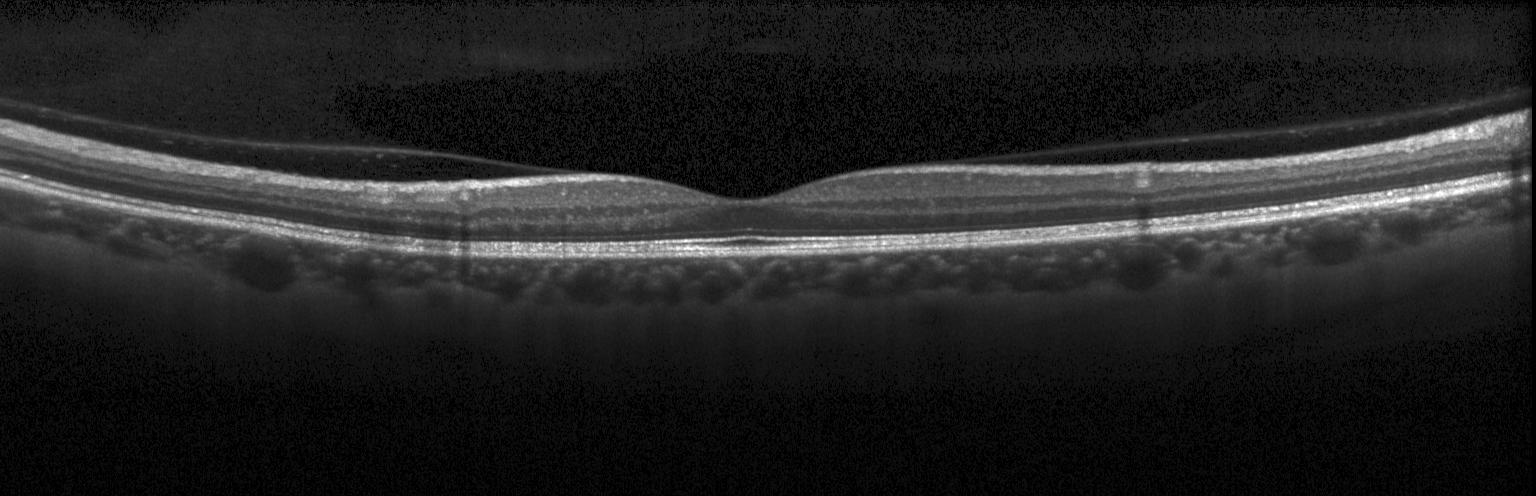

OCT line scan. Finding: no choroidal neovascularization, diabetic macular edema, or drusen.